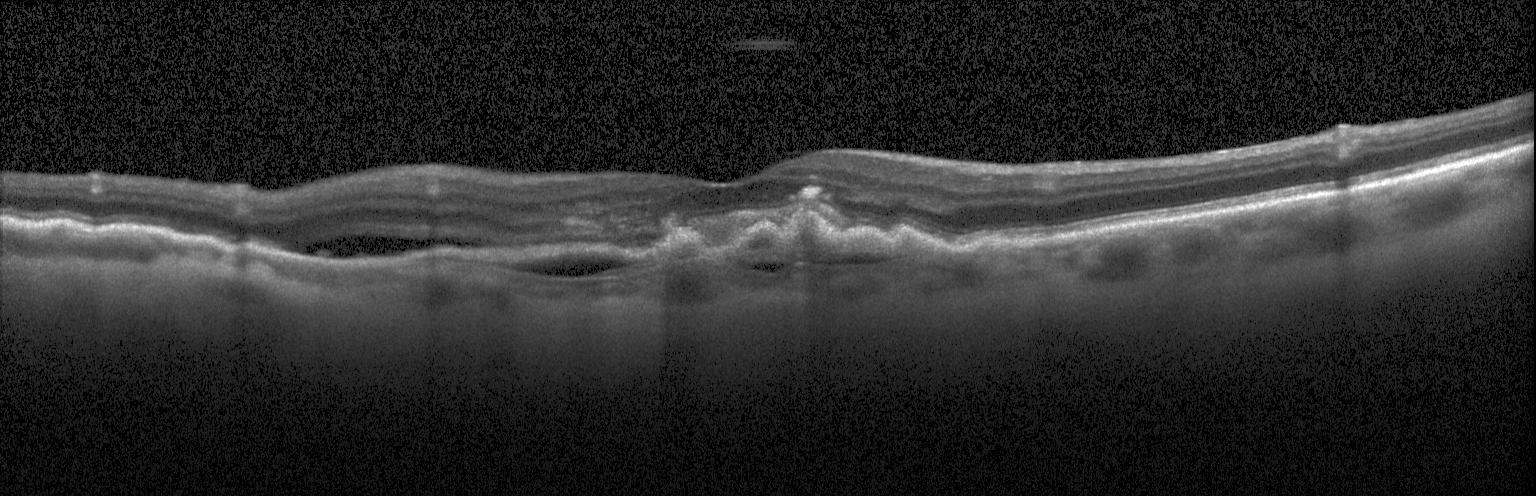 OCT finding: CNV.